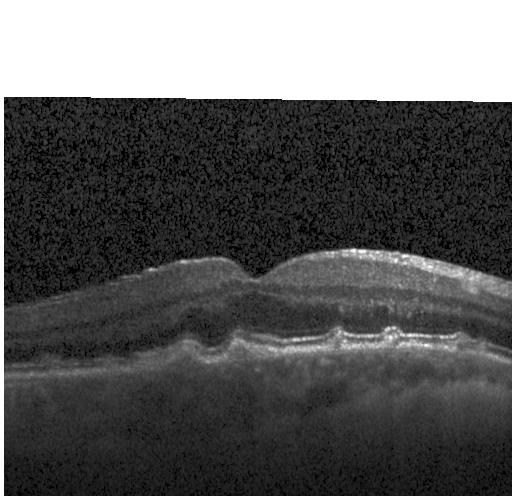 Instrument: Heidelberg Spectralis. Retinal OCT B-scan — Impression: drusen.